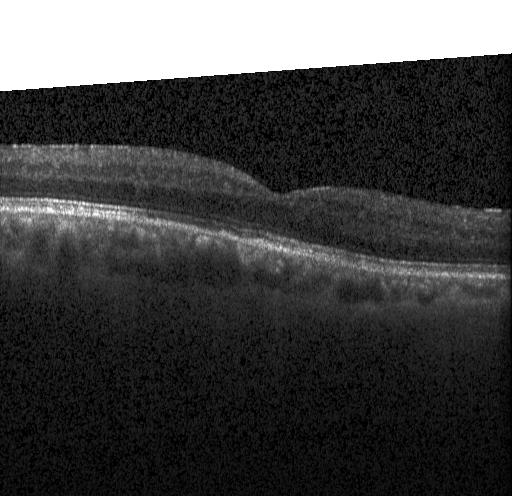
Retinal OCT cross-section; spectral-domain optical coherence tomography.
Macular OCT: no choroidal neovascularization, no diabetic macular edema, and no drusen.